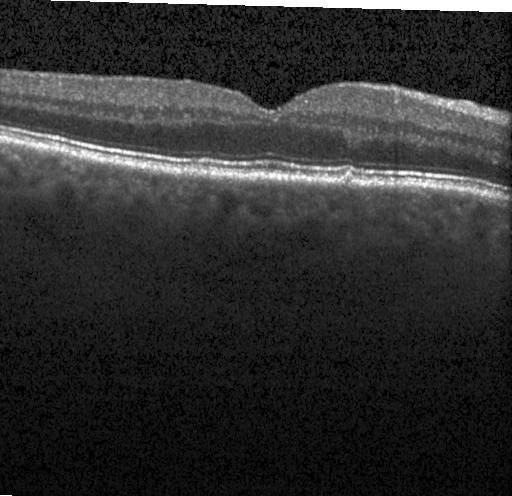 Finding: drusen.